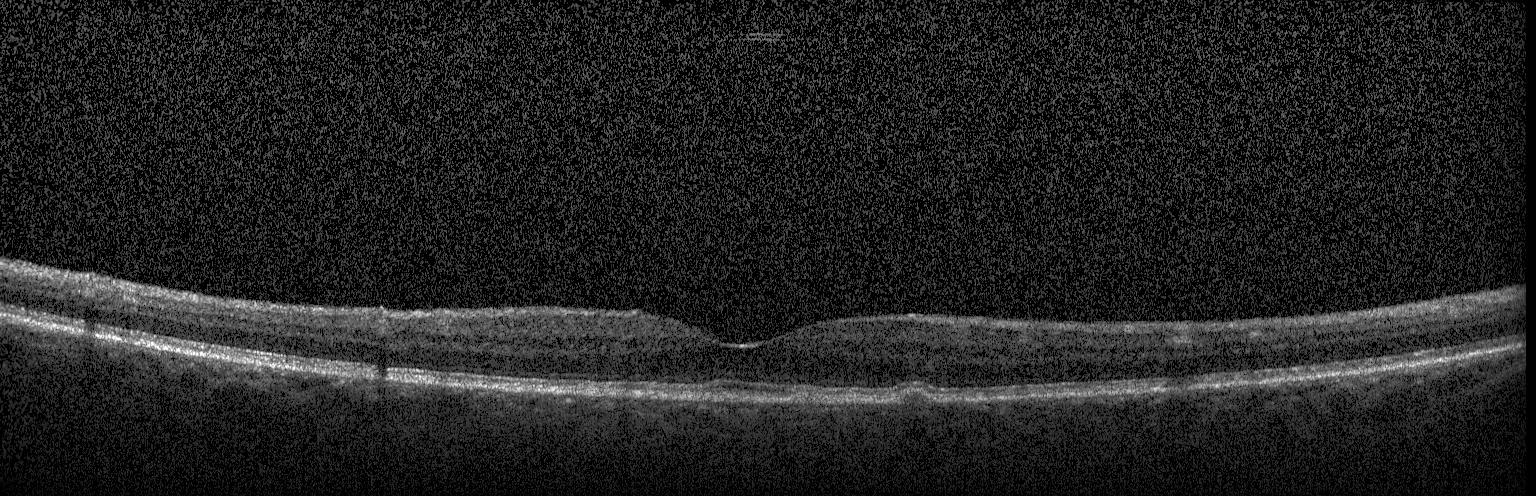
Heidelberg Spectralis. OCT line scan — Finding: multiple drusen.